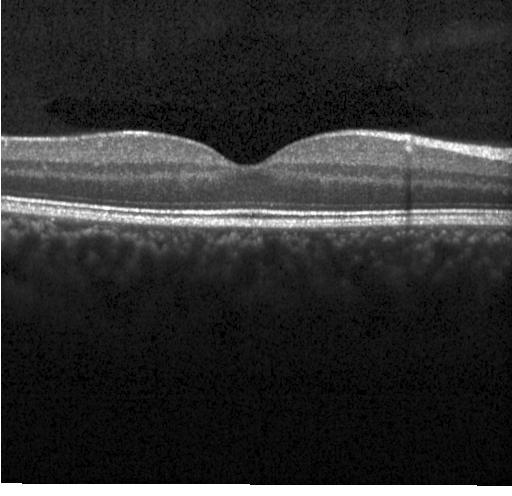 Spectral-domain optical coherence tomography; acquired on a Heidelberg Spectralis; OCT line scan; fovea-centered.
Diagnosis: no choroidal neovascularization, no diabetic macular edema, and no drusen.